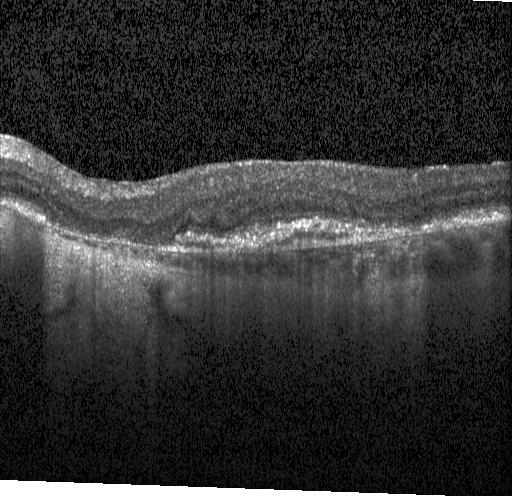 Diagnosis: a choroidal neovascular membrane.